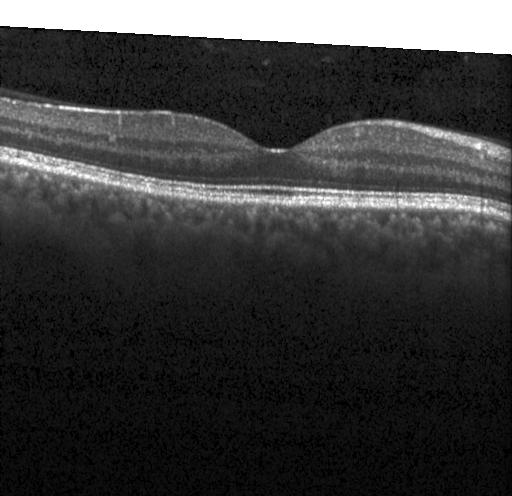 Dx: neither choroidal neovascularization, diabetic macular edema, nor drusen.